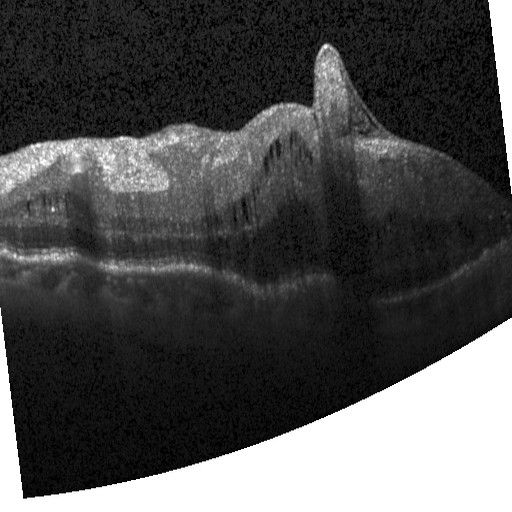
Heidelberg Spectralis, retinal OCT cross-section, spectral-domain OCT — Dx: diabetic macular edema.